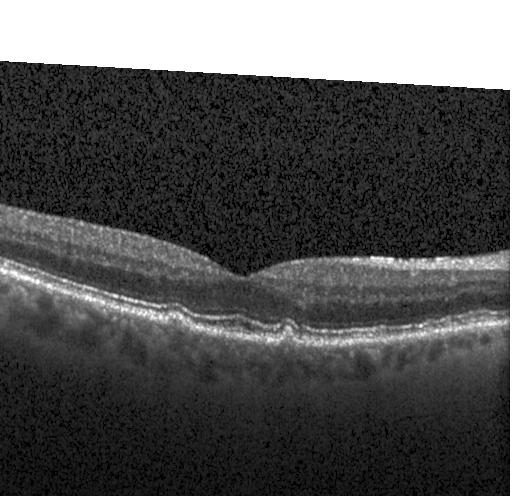
Assessment: sub-RPE drusenoid deposits.